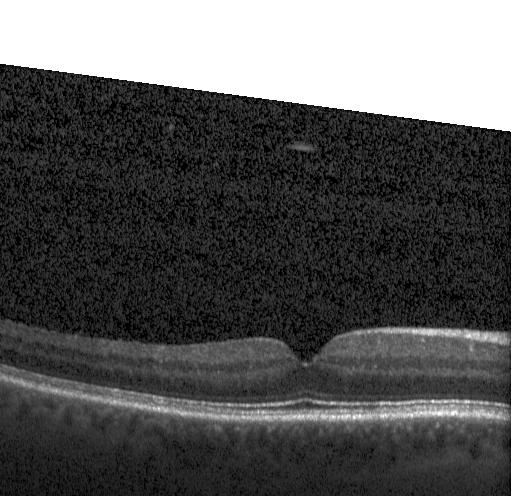 This B-scan demonstrates no choroidal neovascularization, diabetic macular edema, or drusen.